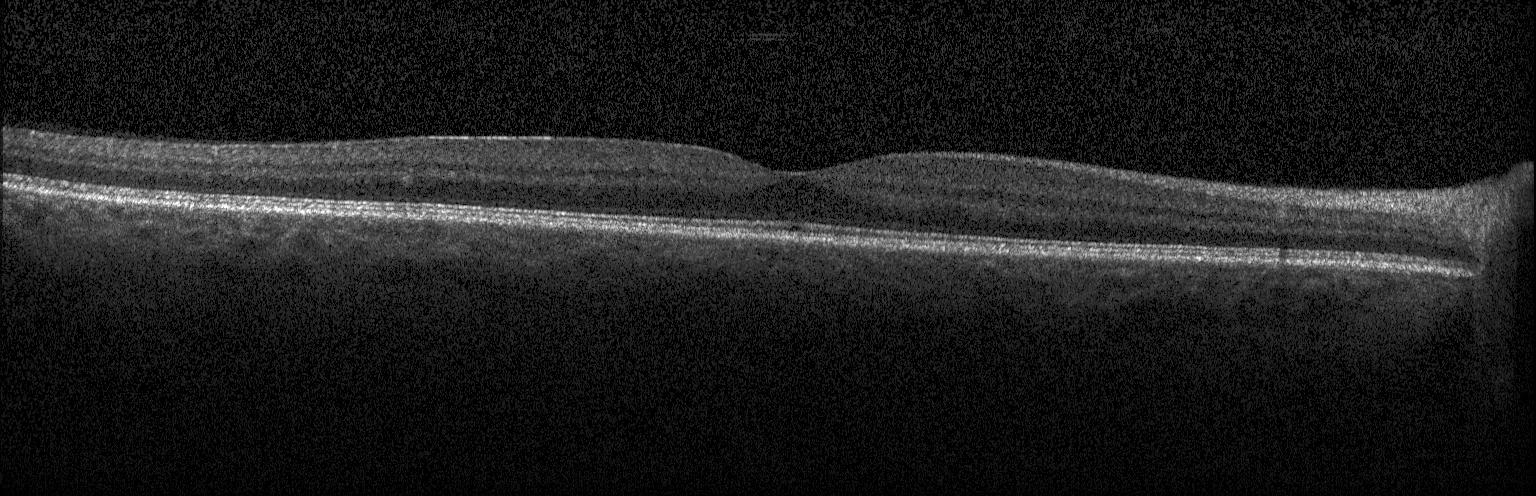
Fovea-centered. OCT line scan. Instrument: Heidelberg Spectralis — Dx: no evidence of CNV, DME, or drusen.